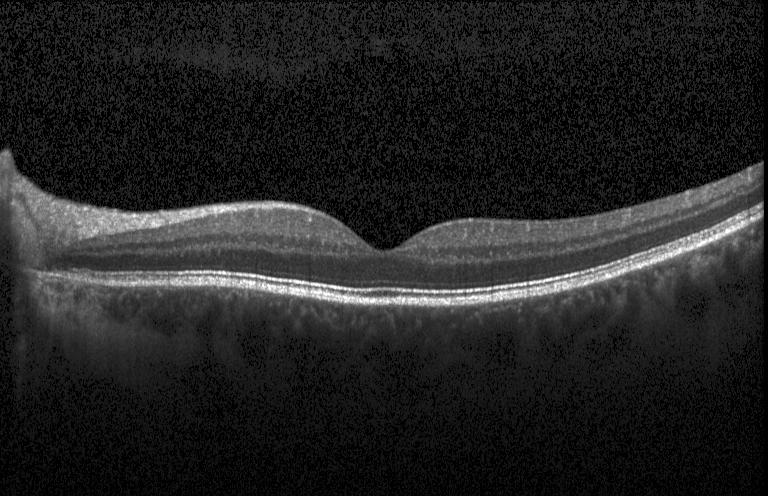

Spectral-domain OCT B-scan: no choroidal neovascularization, no diabetic macular edema, and no drusen.